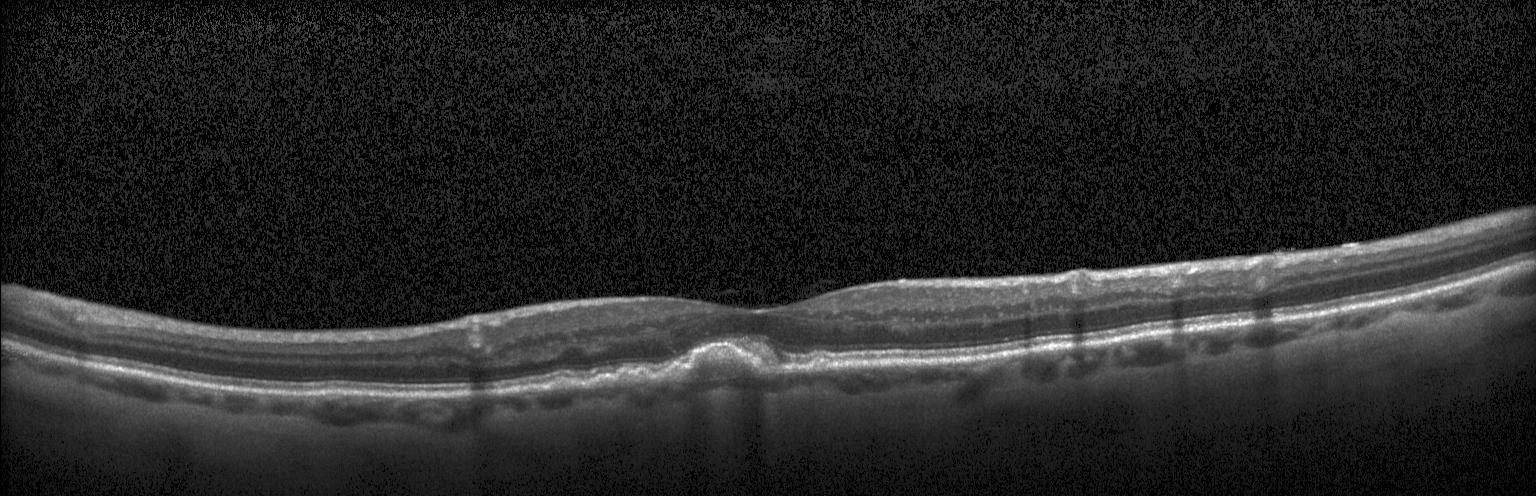
Impression: sub-RPE drusenoid deposits.